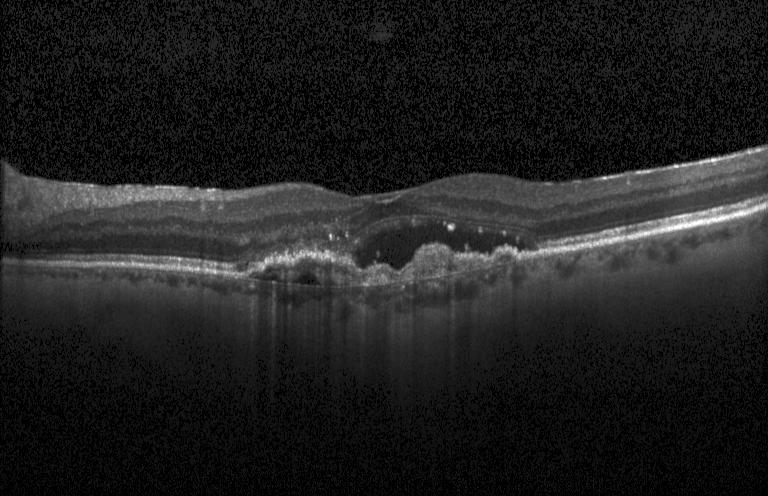
Spectral-domain OCT; optical coherence tomography scan; instrument: Heidelberg Spectralis; fovea-centered.
Diagnosis: a choroidal neovascular membrane.